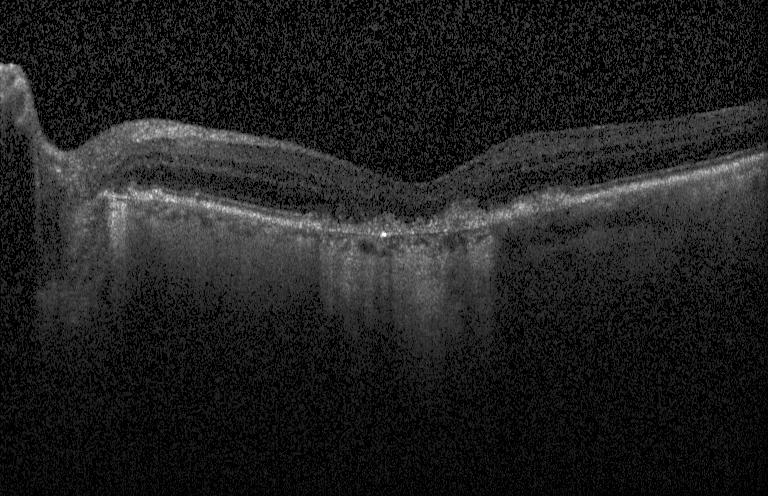 Centered on the fovea, OCT B-scan, spectral-domain optical coherence tomography, Heidelberg Spectralis OCT system — Dx: a choroidal neovascular membrane.